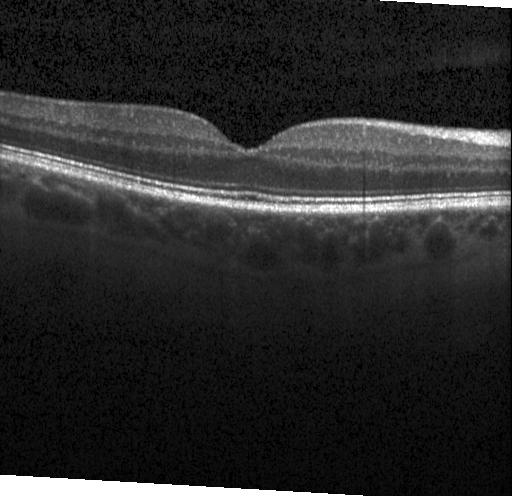

Diagnosis: no choroidal neovascularization, no diabetic macular edema, and no drusen.